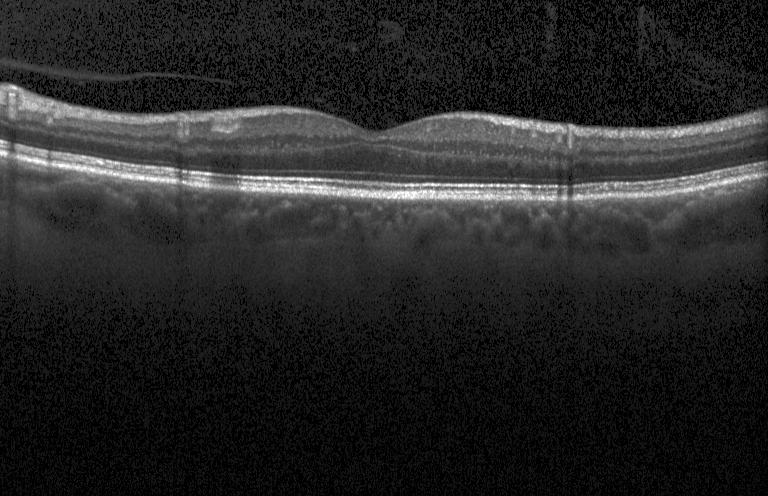 Macular OCT: no choroidal neovascularization, diabetic macular edema, or drusen.